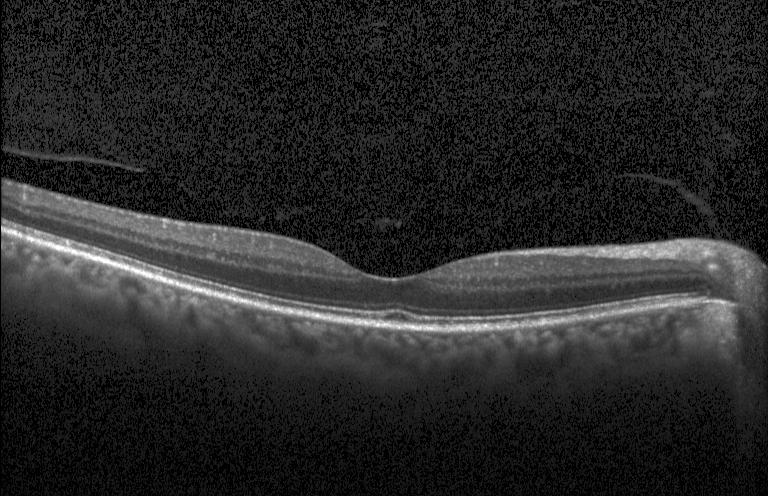
Retinal OCT cross-section showing no choroidal neovascularization, no diabetic macular edema, and no drusen.